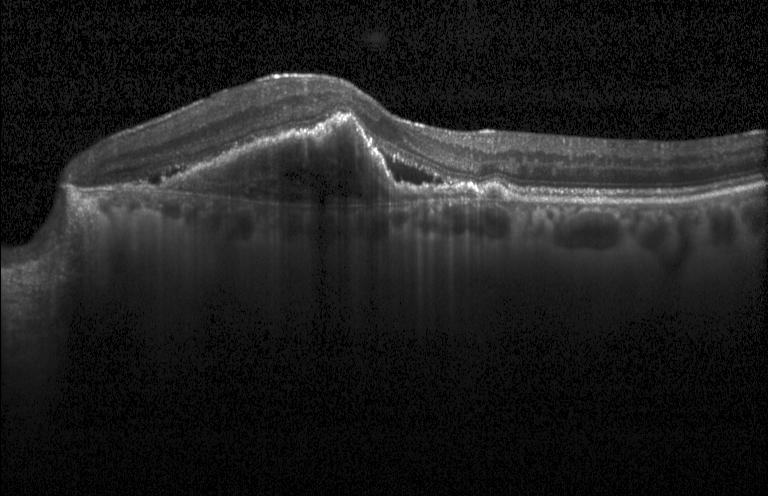

OCT finding: a choroidal neovascular membrane.